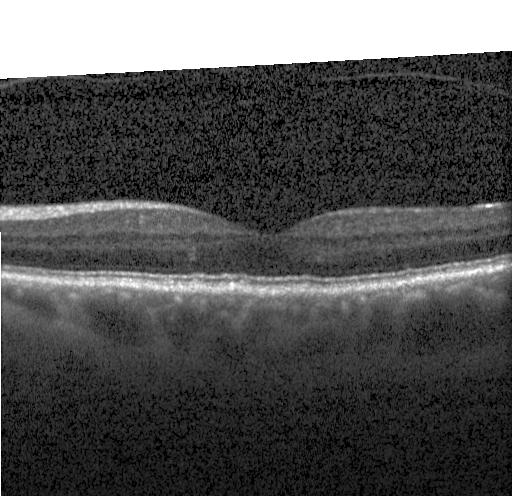
Optical coherence tomography scan; spectral-domain optical coherence tomography. Drusen.